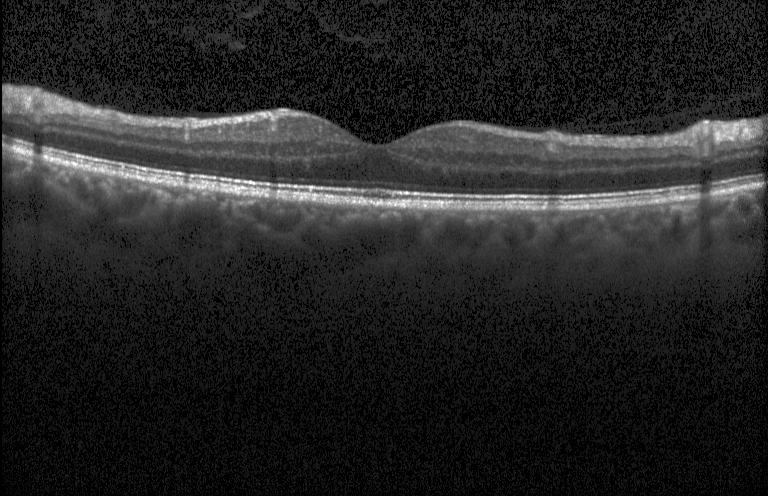 Finding: no CNV, no DME, and no drusen.